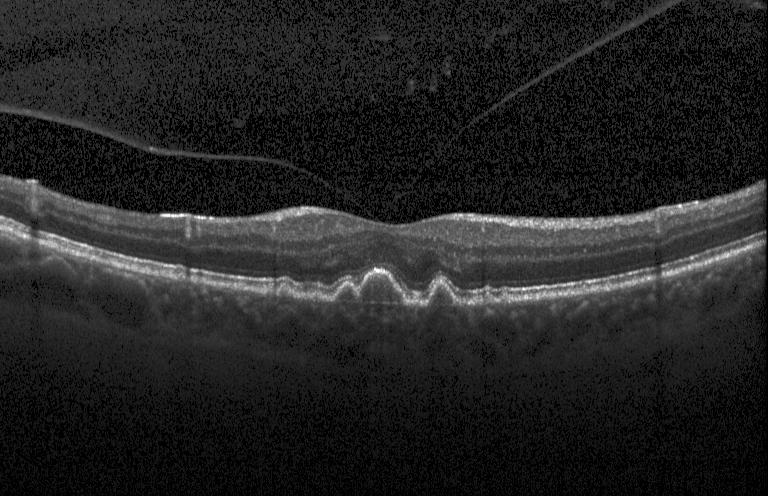
Heidelberg Spectralis OCT system, retinal OCT cross-section, SD-OCT, macular scan
Sub-RPE drusenoid deposits.